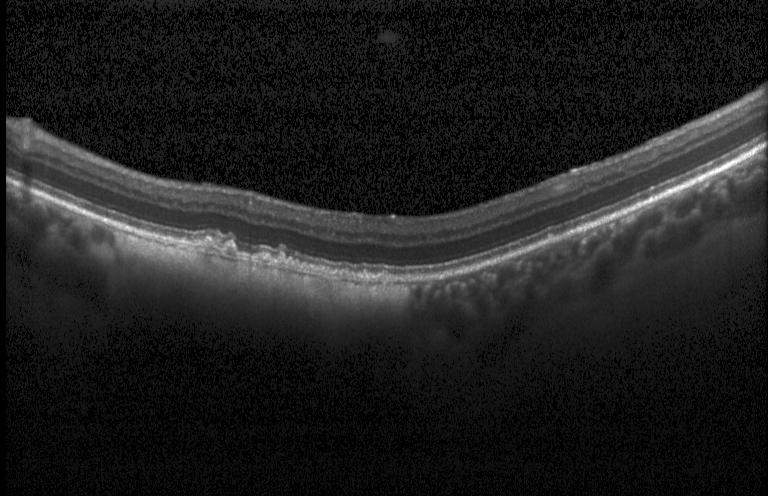 Optical coherence tomography B-scan
This B-scan demonstrates sub-RPE drusenoid deposits.